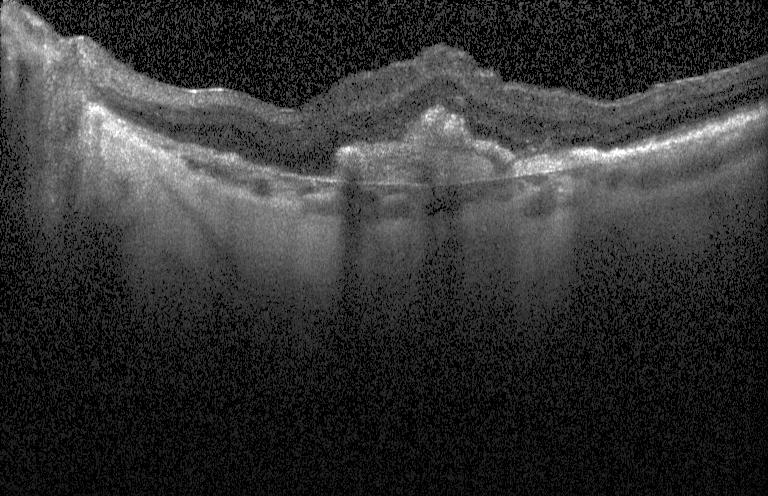 Optical coherence tomography B-scan. Fovea-centered. Impression: a choroidal neovascular membrane.